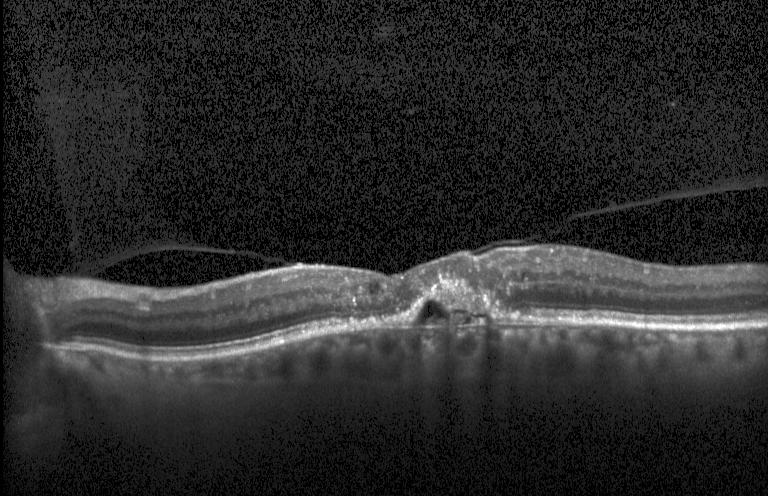

Optical coherence tomography B-scan; Heidelberg Spectralis OCT system; spectral-domain OCT; horizontal scan through the fovea.
Finding: a choroidal neovascular membrane.